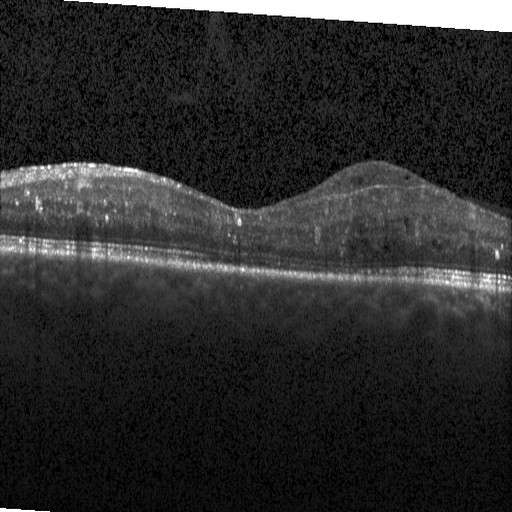

Macular OCT: diabetic macular edema (DME).